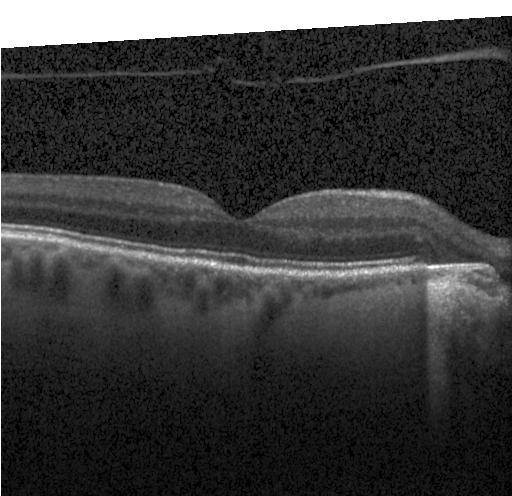 OCT line scan.
Finding: neither choroidal neovascularization, diabetic macular edema, nor drusen.